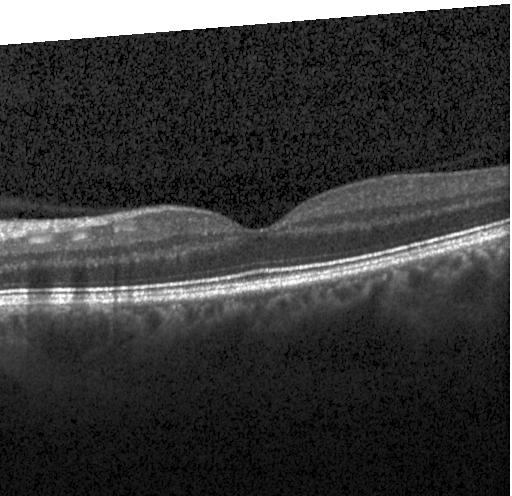
Dx: no evidence of choroidal neovascularization, diabetic macular edema, or drusen.